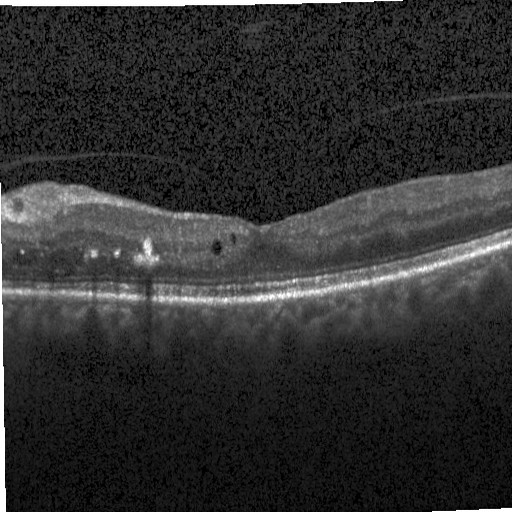
Optical coherence tomography B-scan.
Macular OCT: DME.